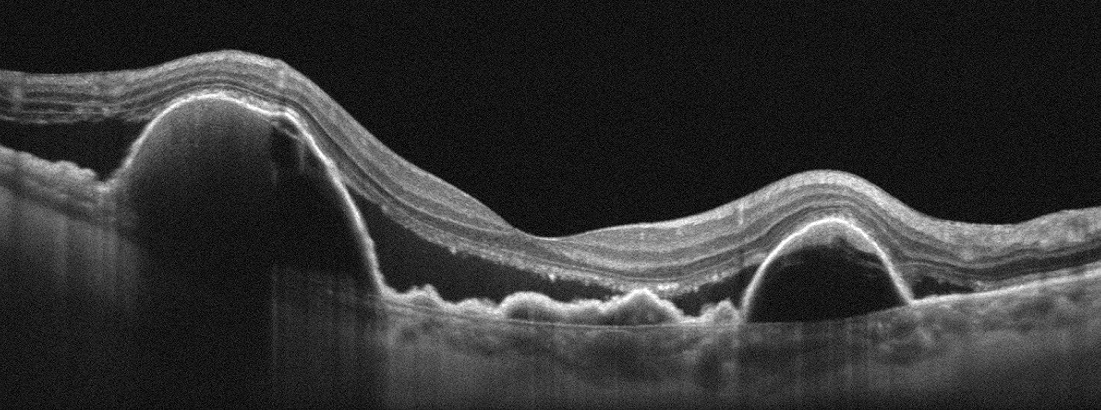 Impression: age-related macular degeneration.